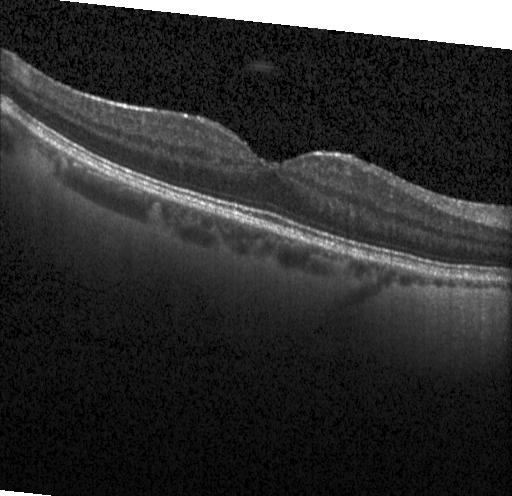

Retinal OCT cross-section showing no evidence of CNV, DME, or drusen.